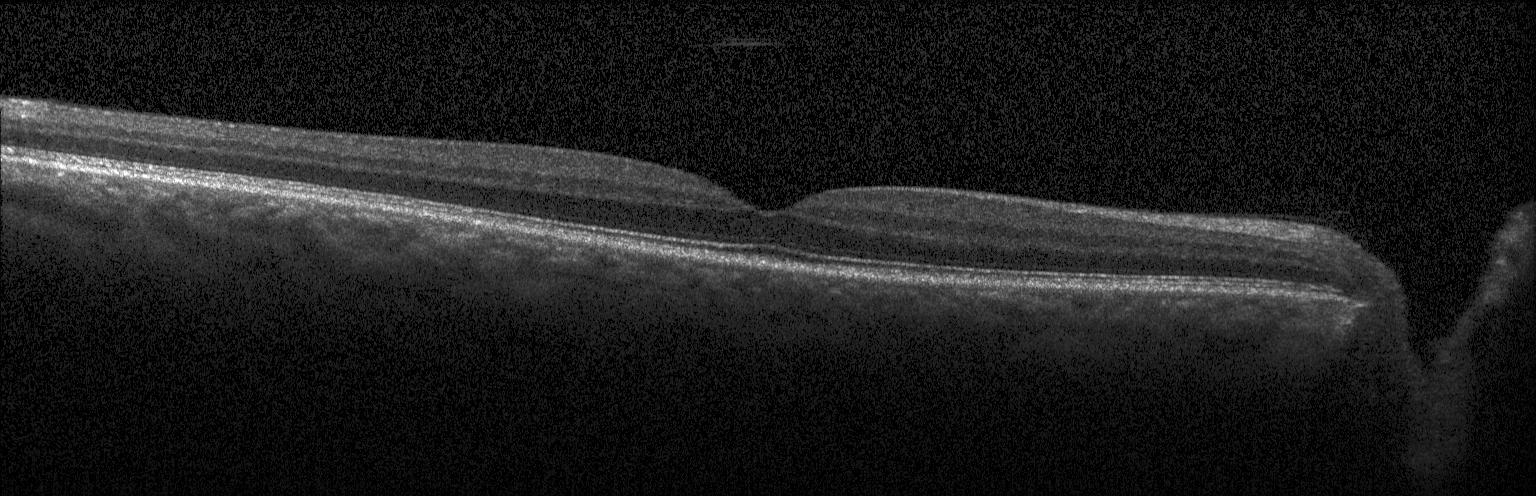 Dx: neither choroidal neovascularization, diabetic macular edema, nor drusen.